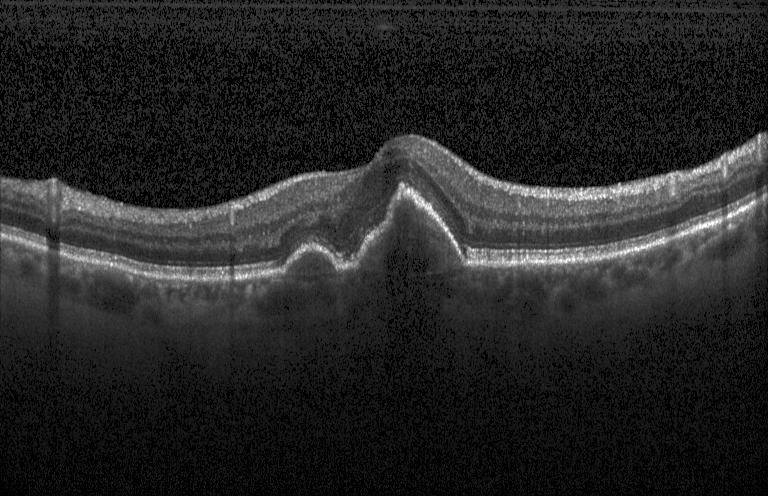

Finding: choroidal neovascularization.